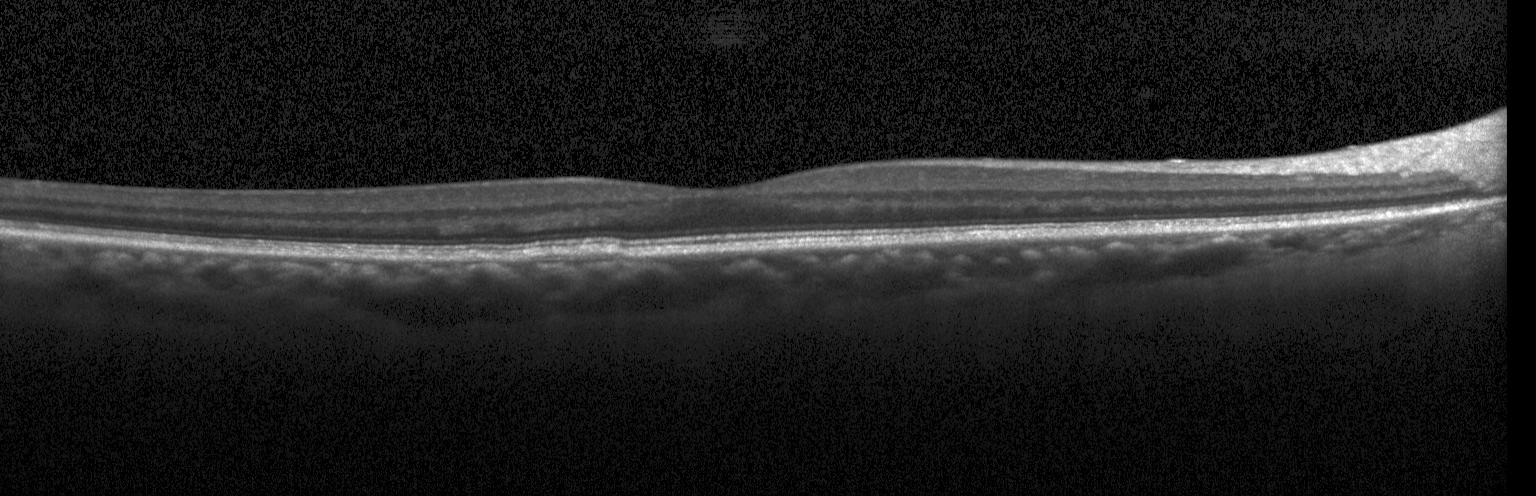 Spectral-domain OCT · horizontal scan through the fovea · Heidelberg Spectralis OCT system · optical coherence tomography B-scan
Macular OCT: no evidence of CNV, DME, or drusen.